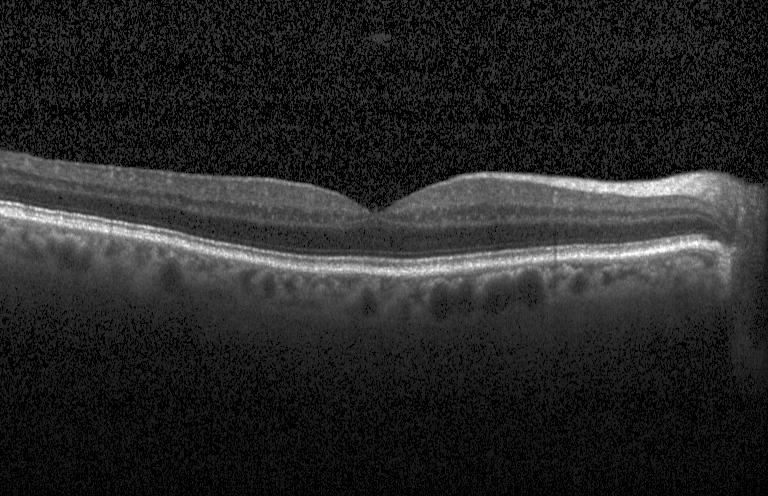

Retinal OCT cross-section · Heidelberg Spectralis
The scan shows neither choroidal neovascularization, diabetic macular edema, nor drusen.